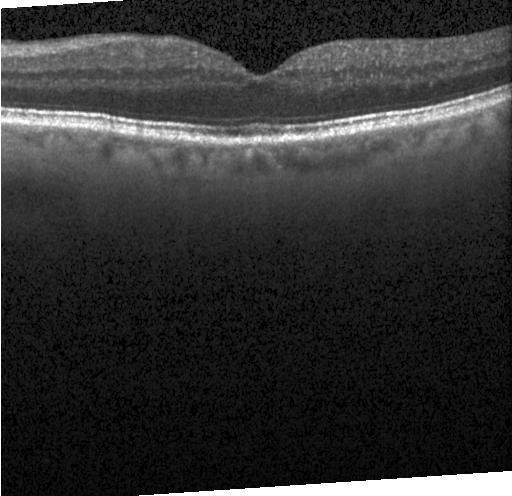
Diagnosis: no choroidal neovascularization, diabetic macular edema, or drusen.